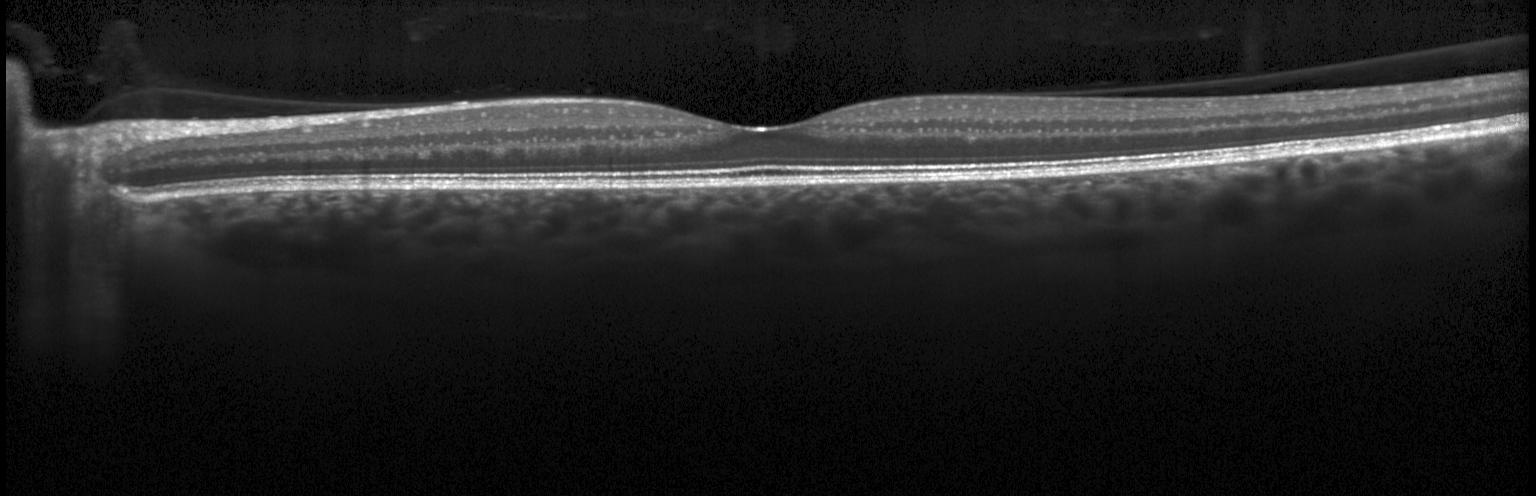 Spectral-domain OCT · instrument: Heidelberg Spectralis · retinal OCT B-scan
Assessment: no choroidal neovascularization, diabetic macular edema, or drusen.